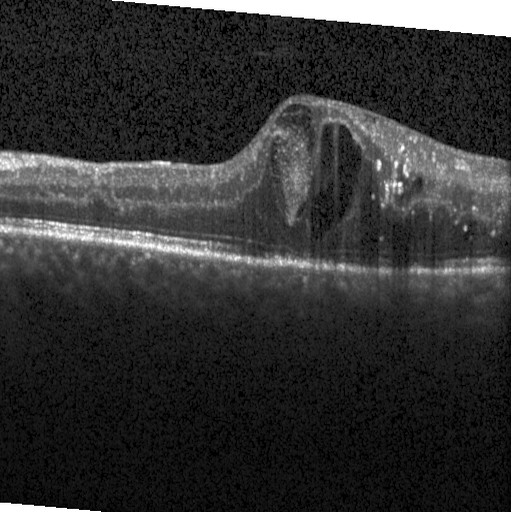 Finding: diabetic macular edema (DME).